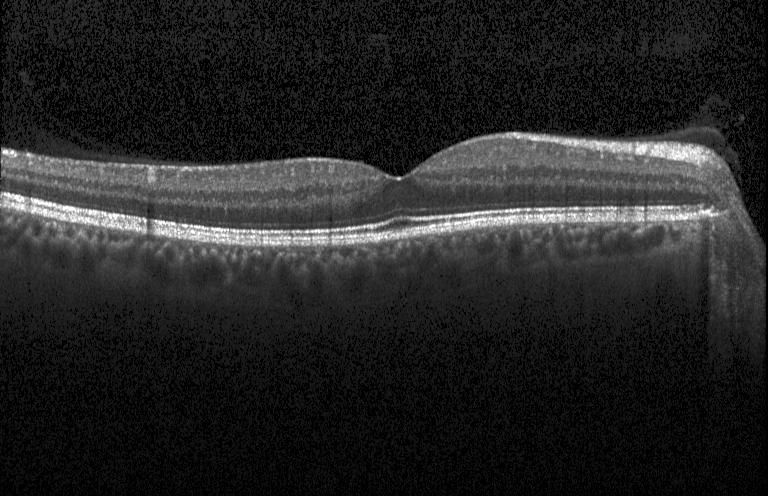
Spectral-domain OCT, optical coherence tomography scan. Impression: no CNV, DME, or drusen.